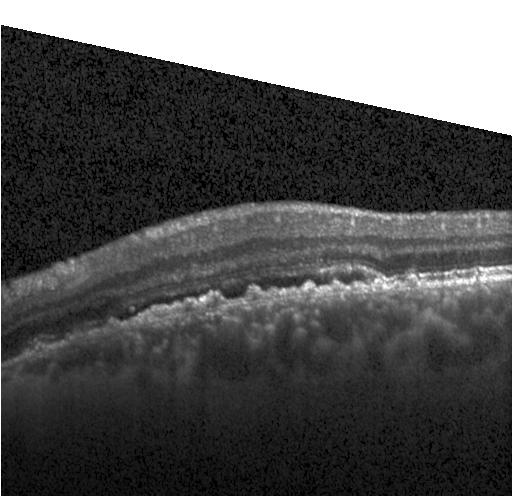 Optical coherence tomography scan.
Choroidal neovascularization.